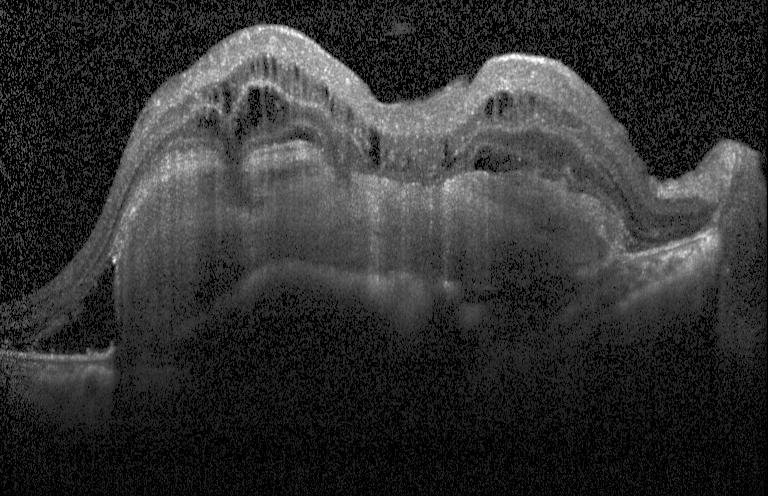

OCT line scan.
Assessment: CNV.